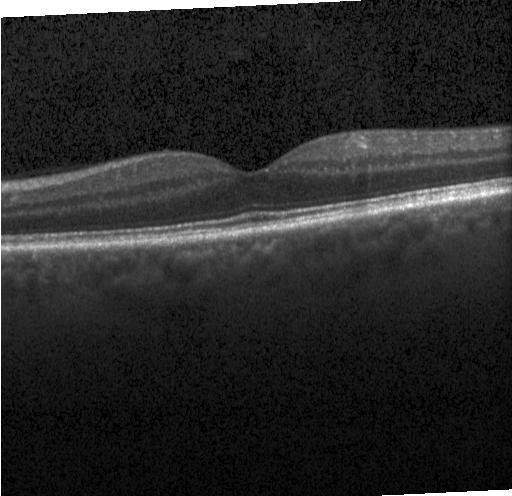
Retinal OCT cross-section showing neither choroidal neovascularization, diabetic macular edema, nor drusen.